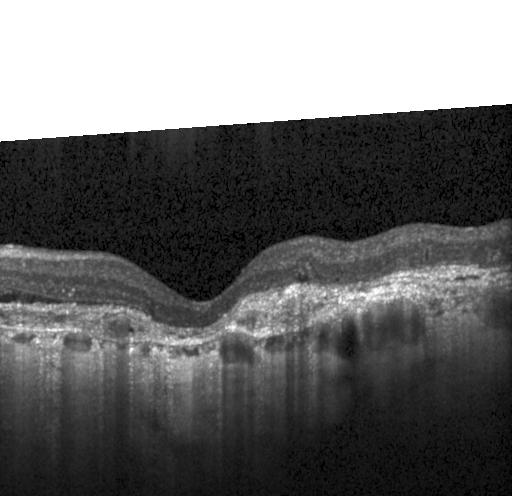
Retinal OCT B-scan. Heidelberg Spectralis OCT system. SD-OCT. Finding: a choroidal neovascular membrane.